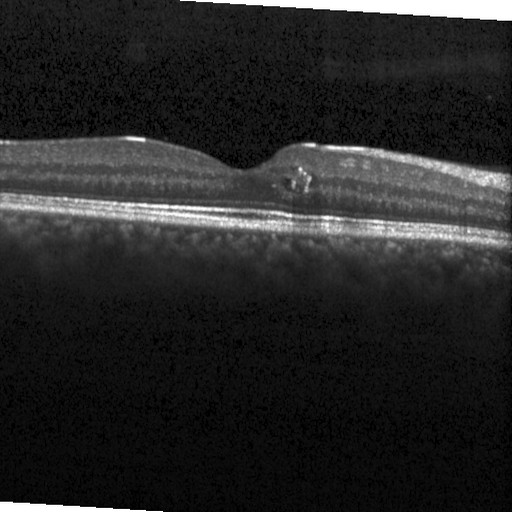

Dx: diabetic macular edema.